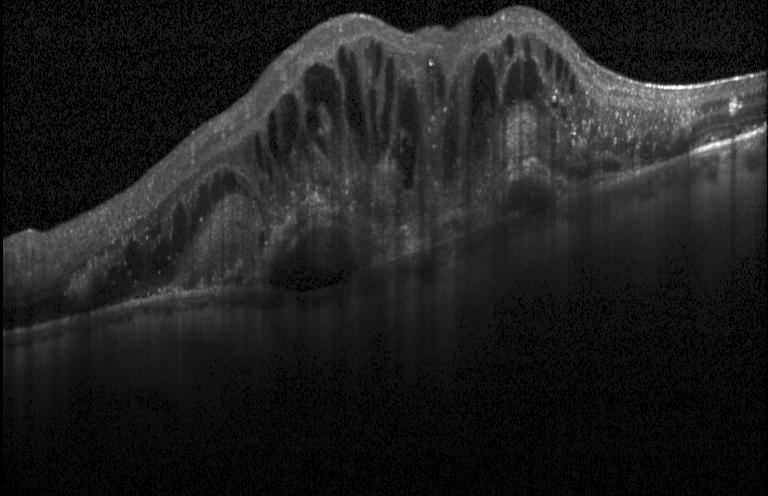 SD-OCT, retinal OCT B-scan — This B-scan demonstrates choroidal neovascularization.